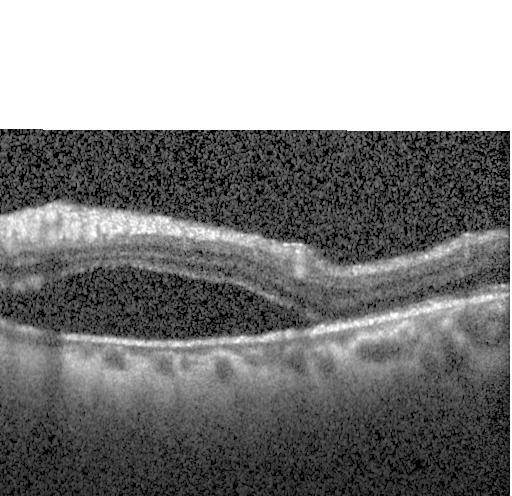 Spectral-domain OCT B-scan: choroidal neovascularization.